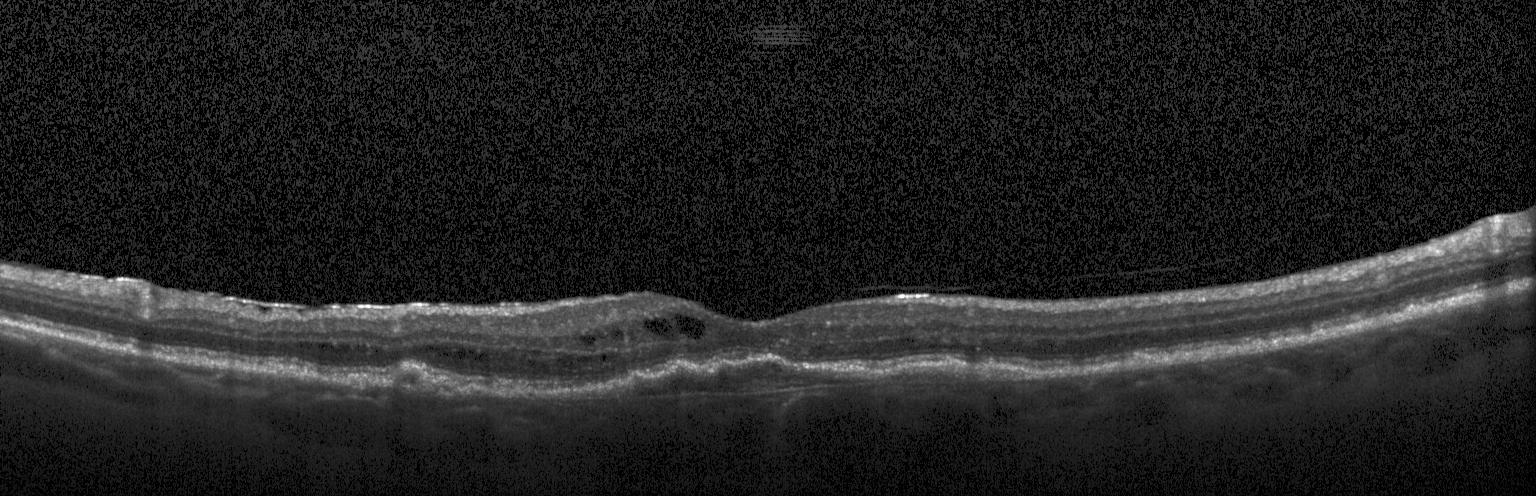 Finding: choroidal neovascularization (CNV).